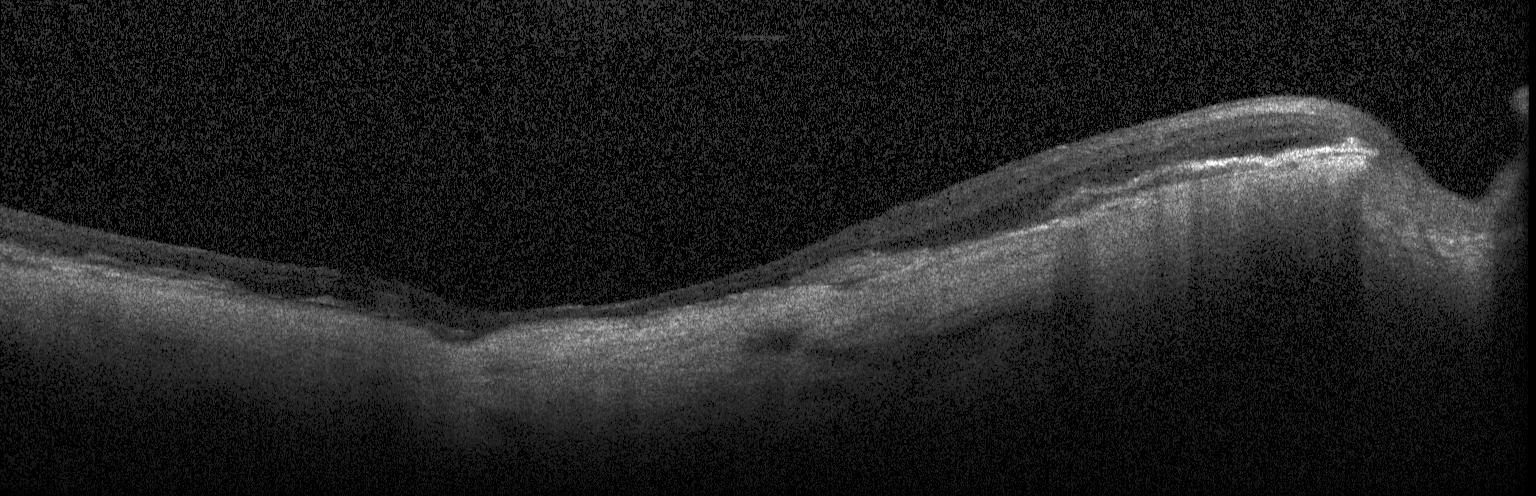
Optical coherence tomography B-scan — Finding: a choroidal neovascular membrane.